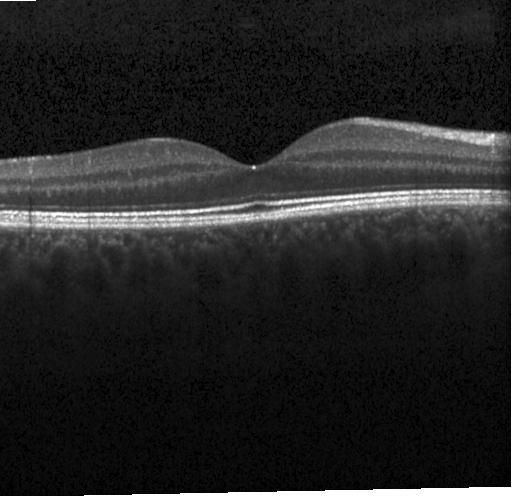

Centered on the fovea. OCT line scan. OCT finding: no CNV, no DME, and no drusen.